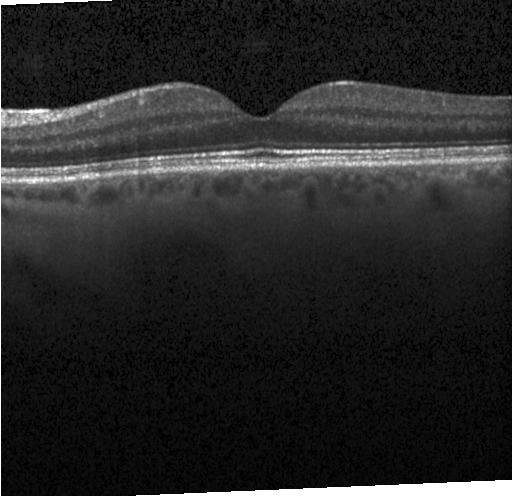
Retinal OCT cross-section. Dx: no choroidal neovascularization, no diabetic macular edema, and no drusen.